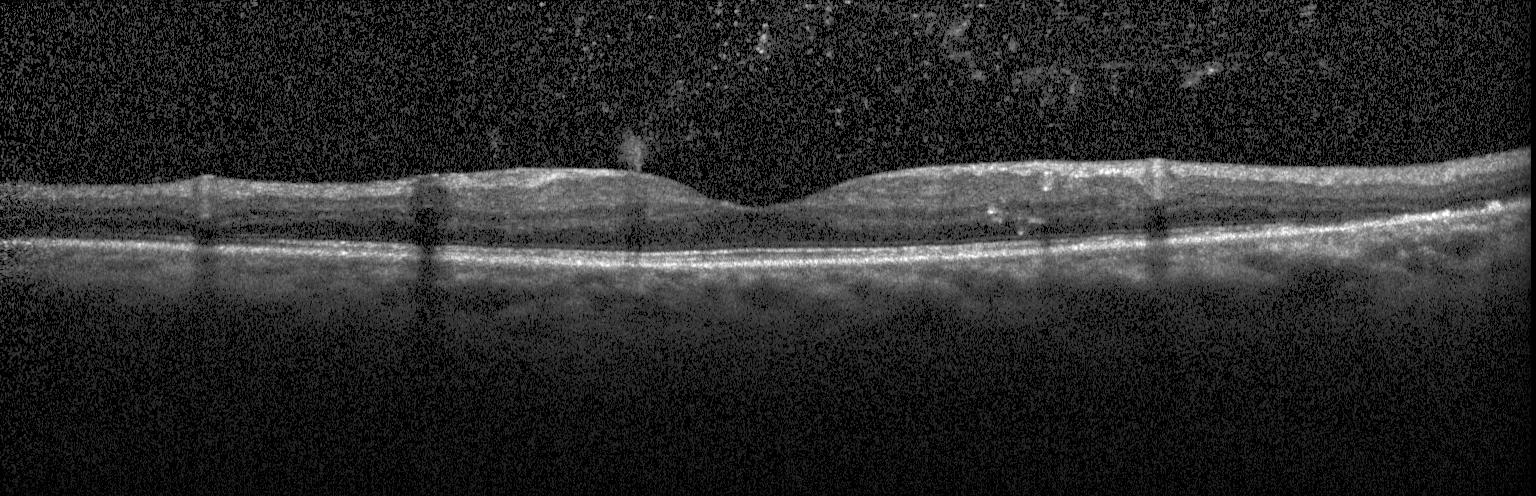
Finding: diabetic macular edema.